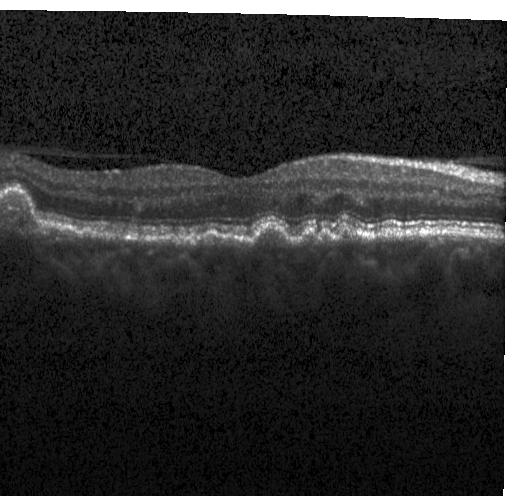

OCT line scan. This B-scan demonstrates multiple drusen.